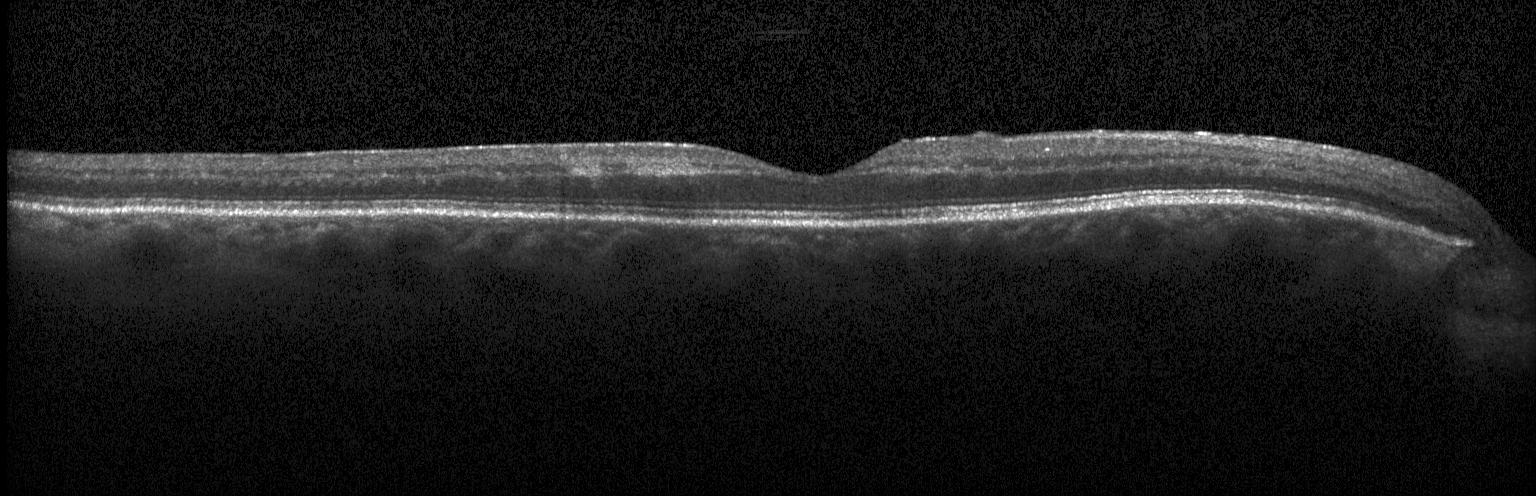

Through the macula. Optical coherence tomography scan. Spectral-domain OCT. Instrument: Heidelberg Spectralis.
This B-scan demonstrates no choroidal neovascularization, diabetic macular edema, or drusen.